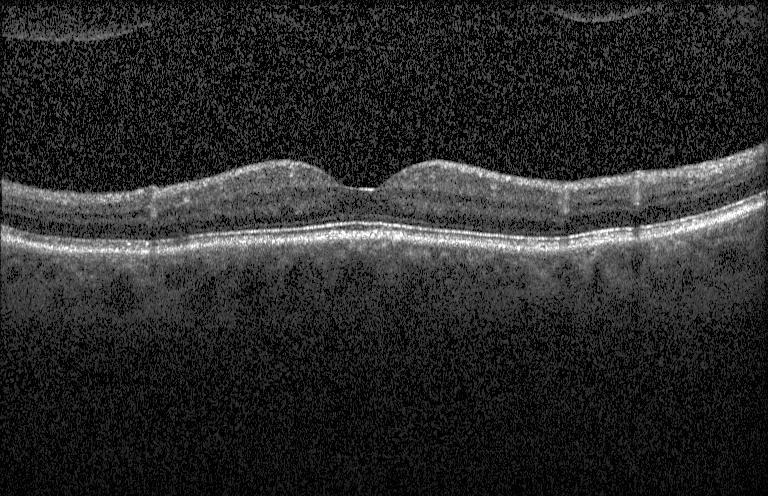 Optical coherence tomography B-scan — Finding: no evidence of choroidal neovascularization, diabetic macular edema, or drusen.